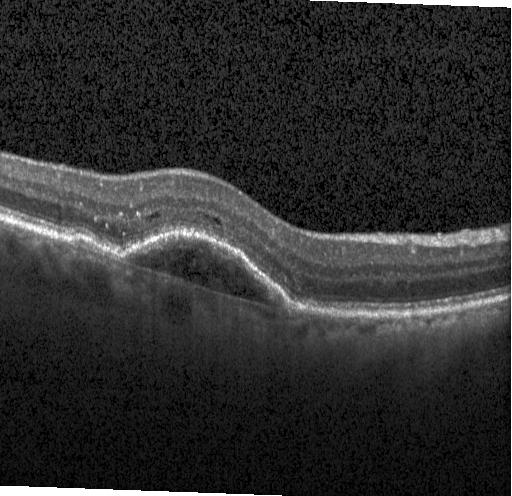 Fovea-centered, instrument: Heidelberg Spectralis, optical coherence tomography scan
CNV.